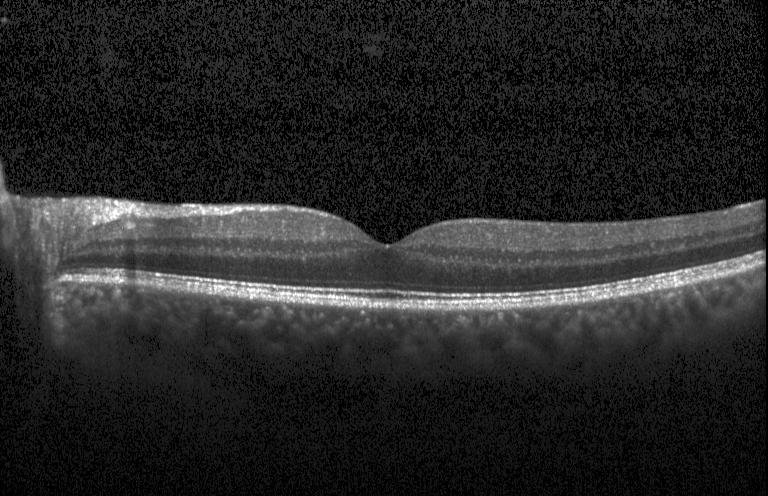 The scan shows no choroidal neovascularization, no diabetic macular edema, and no drusen.